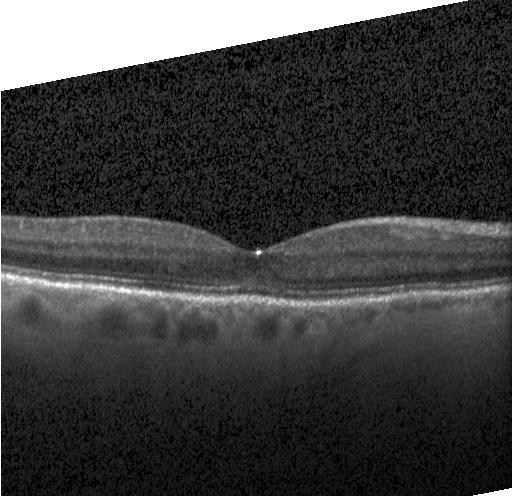
Through the macula, retinal OCT B-scan — Finding: no evidence of choroidal neovascularization, diabetic macular edema, or drusen.